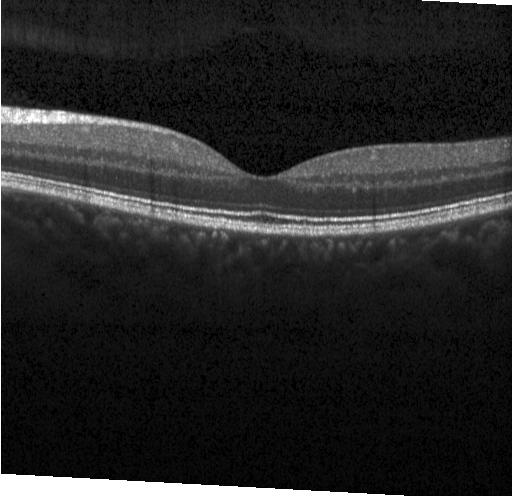

Macular OCT: neither CNV, DME, nor drusen.